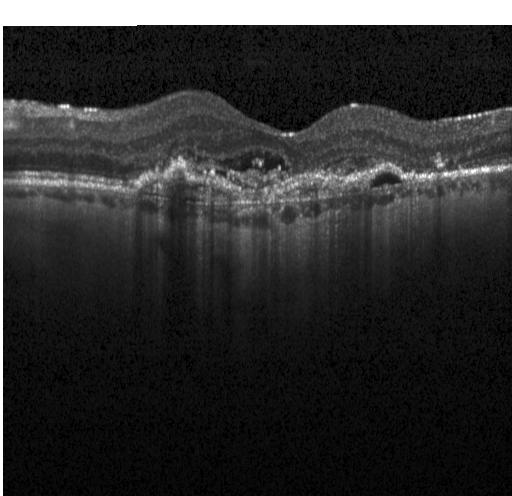 Spectral-domain OCT, OCT B-scan, centered on the fovea
Diagnosis: a choroidal neovascular membrane.